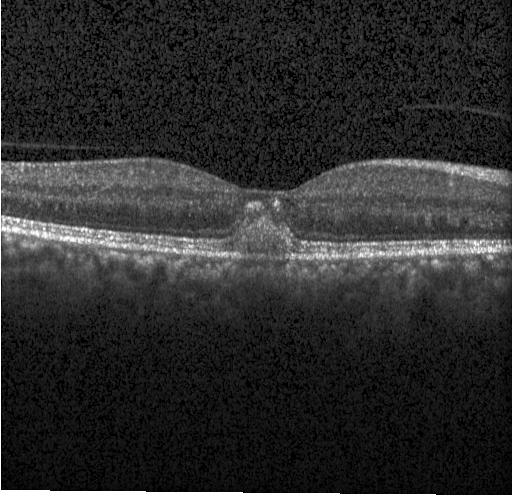 Diagnosis: a choroidal neovascular membrane.